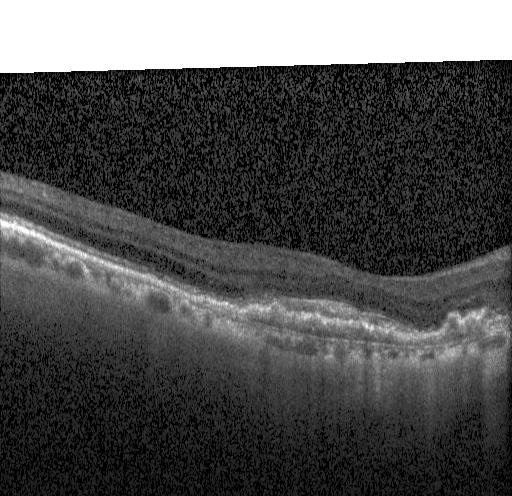

OCT line scan — This B-scan demonstrates a choroidal neovascular membrane.